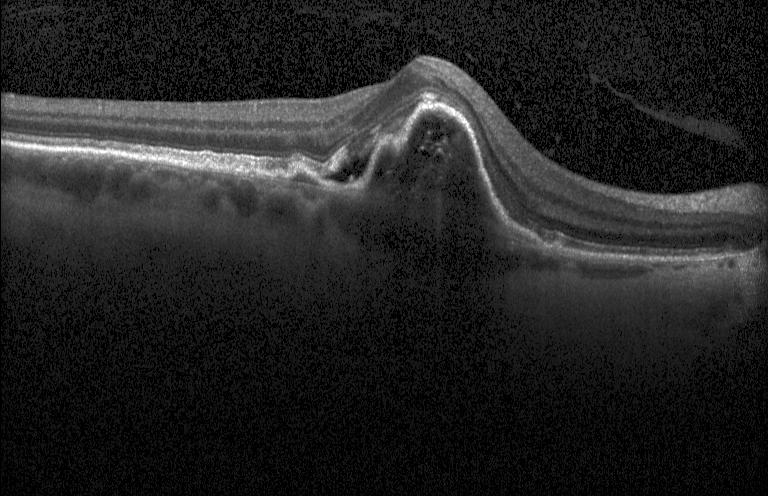 Finding: a choroidal neovascular membrane.